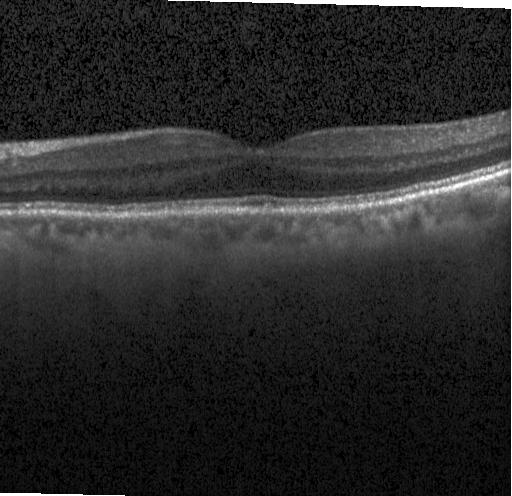 Impression: neither CNV, DME, nor drusen.